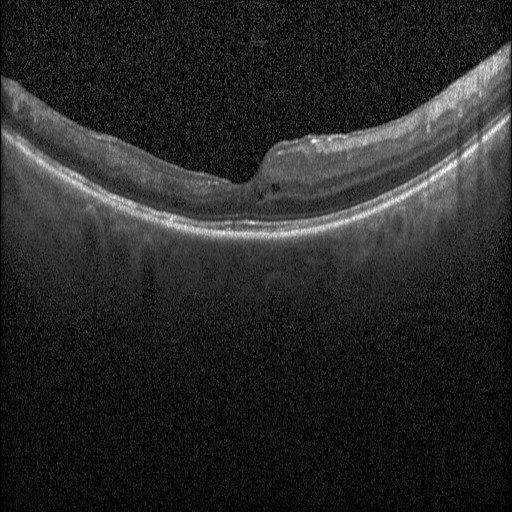
This B-scan demonstrates DME.